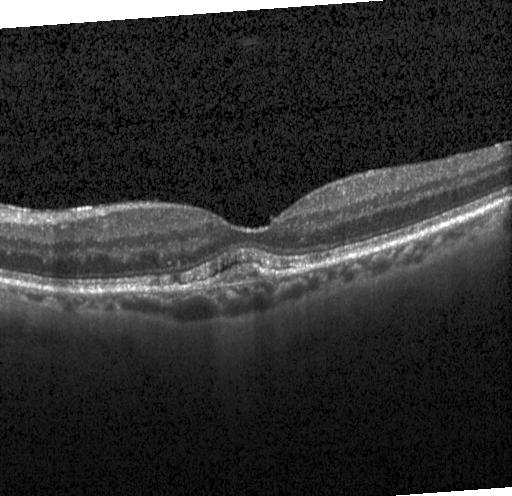 Instrument: Heidelberg Spectralis; fovea-centered; optical coherence tomography B-scan — Diagnosis: a choroidal neovascular membrane.